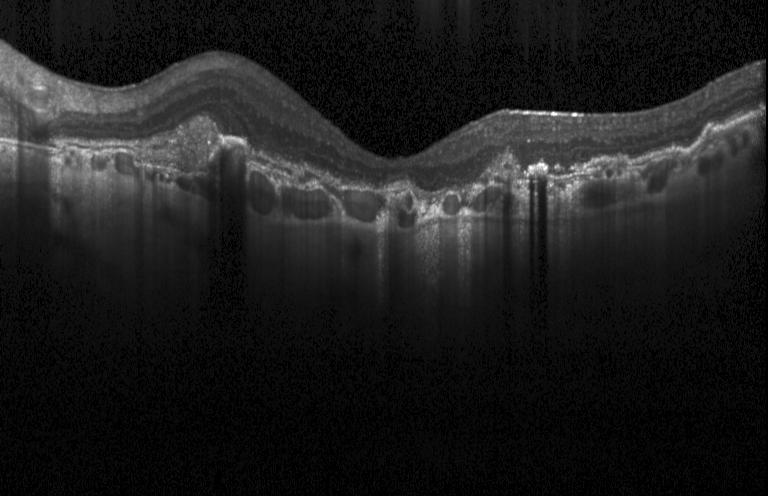

Centered on the fovea. OCT line scan — Impression: CNV.